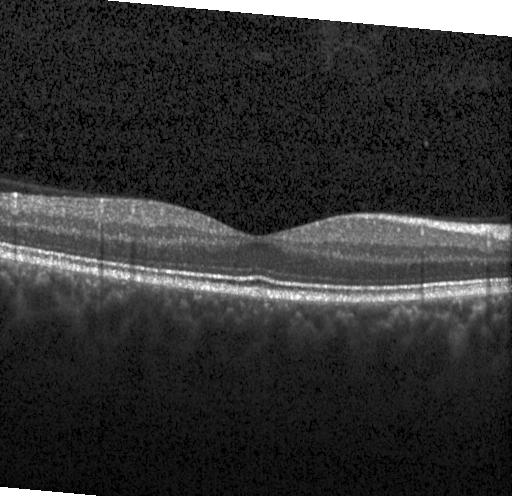 Dx: neither choroidal neovascularization, diabetic macular edema, nor drusen.